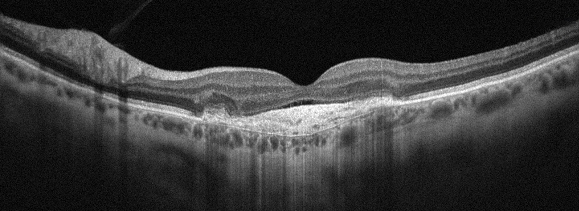 OS. OCT B-scan. Fovea-centered. Instrument: Optovue Avanti RTVue XR.
Impression: age-related macular degeneration (AMD).